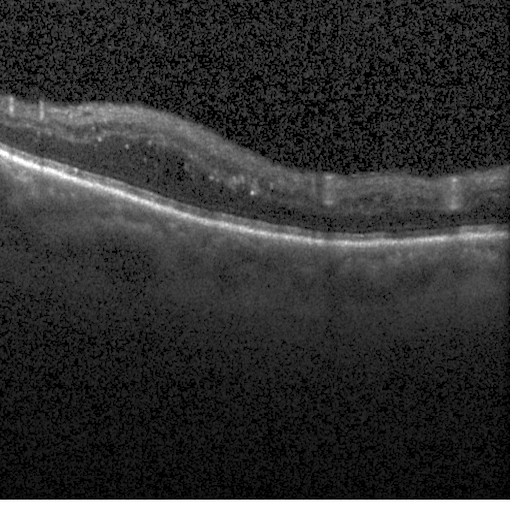

OCT B-scan · fovea-centered
Finding: diabetic macular edema (DME).